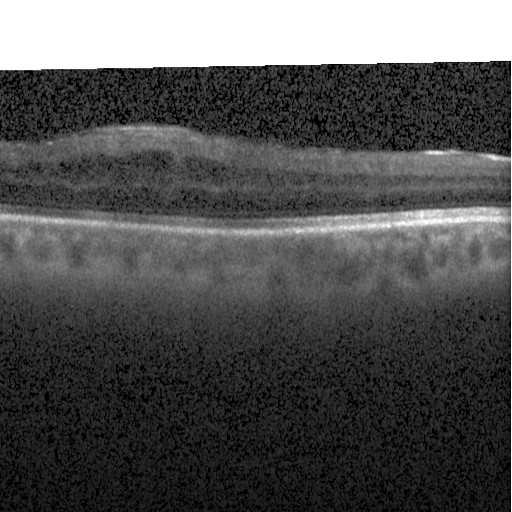
Spectral-domain OCT, horizontal scan through the fovea, retinal OCT B-scan. This B-scan demonstrates diabetic macular edema (DME).